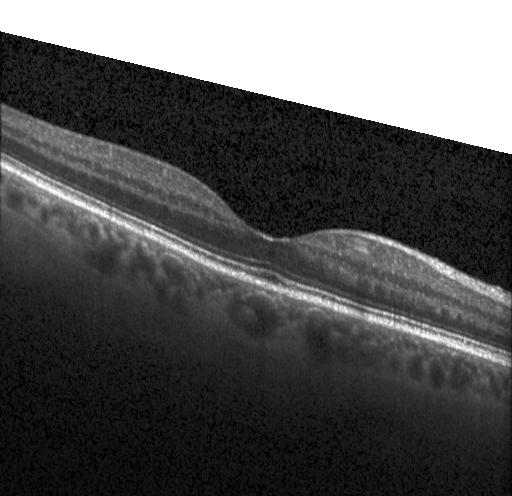
Macular OCT: no choroidal neovascularization, no diabetic macular edema, and no drusen.